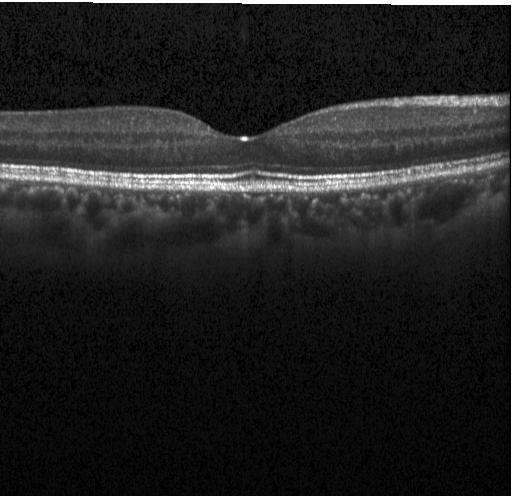

Through the macula; OCT line scan; Heidelberg Spectralis OCT system; spectral-domain optical coherence tomography. Impression: no evidence of CNV, DME, or drusen.